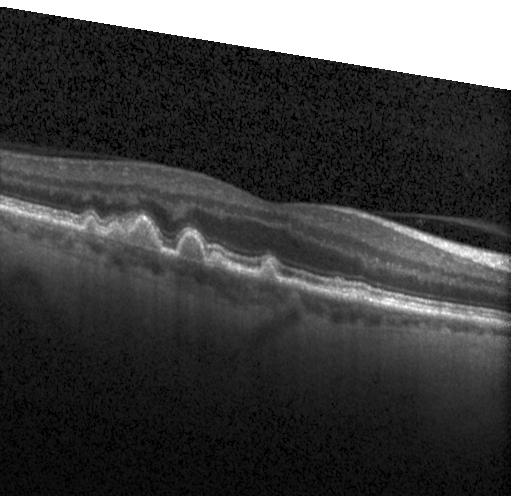

Heidelberg Spectralis OCT system; SD-OCT; optical coherence tomography B-scan
Dx: sub-RPE drusenoid deposits.